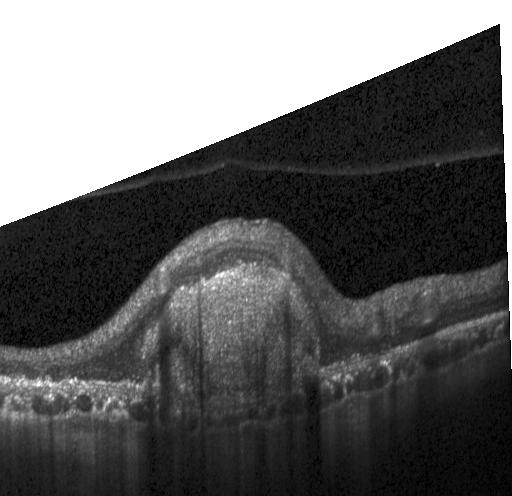 Diagnosis: a choroidal neovascular membrane.